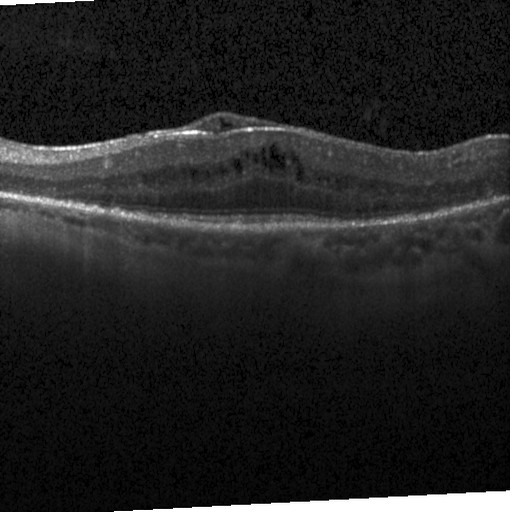

Dx: diabetic macular edema (DME).